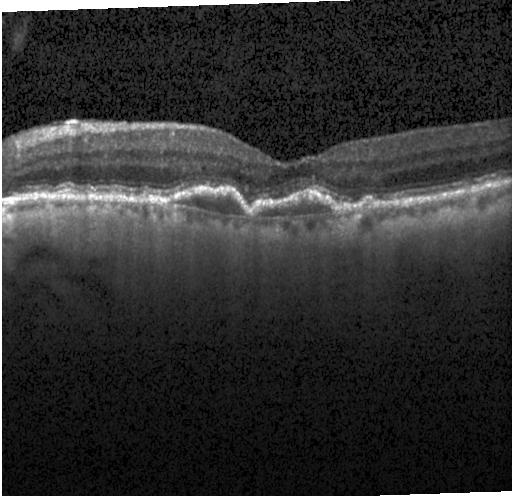

Optical coherence tomography B-scan. This B-scan demonstrates choroidal neovascularization.